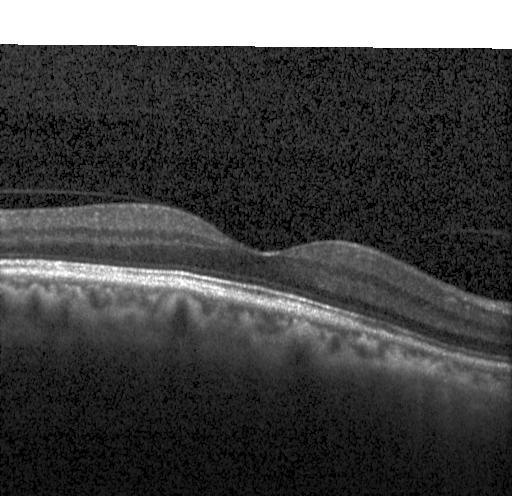
OCT line scan · through the macula · SD-OCT · instrument: Heidelberg Spectralis. Finding: no choroidal neovascularization, diabetic macular edema, or drusen.